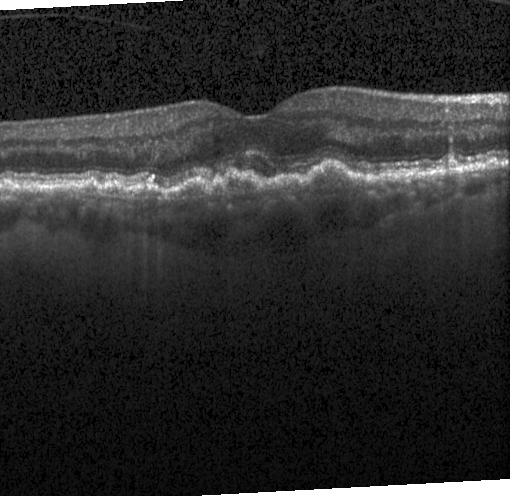

OCT B-scan showing a choroidal neovascular membrane.